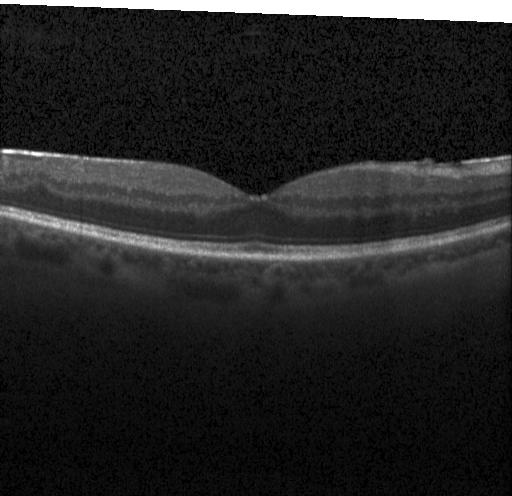

Finding: no choroidal neovascularization, no diabetic macular edema, and no drusen.